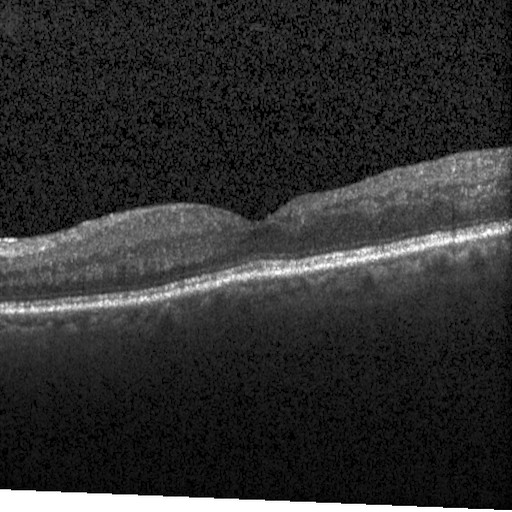 Instrument: Heidelberg Spectralis, optical coherence tomography B-scan.
Diagnosis: diabetic macular edema.